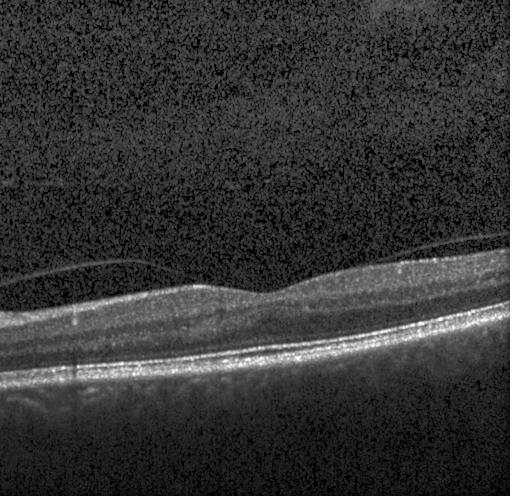

Assessment: no CNV, DME, or drusen.